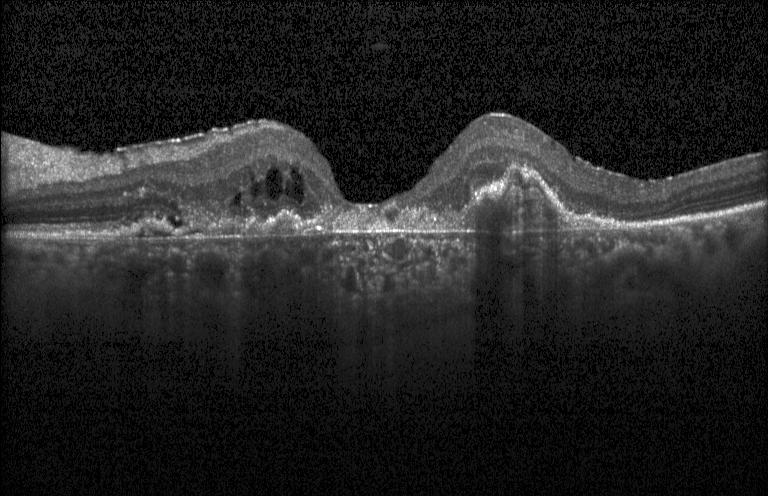

SD-OCT · optical coherence tomography B-scan.
A choroidal neovascular membrane.